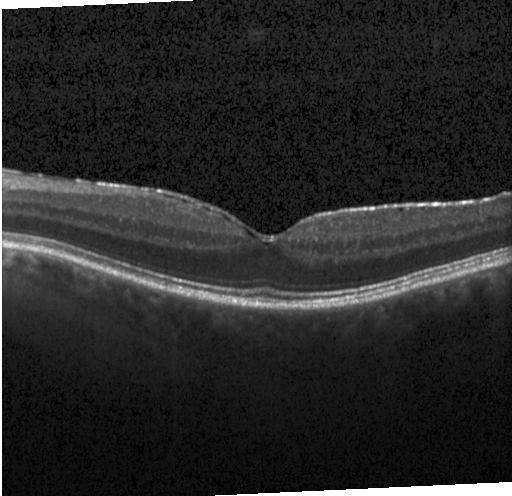
OCT B-scan
OCT finding: neither choroidal neovascularization, diabetic macular edema, nor drusen.